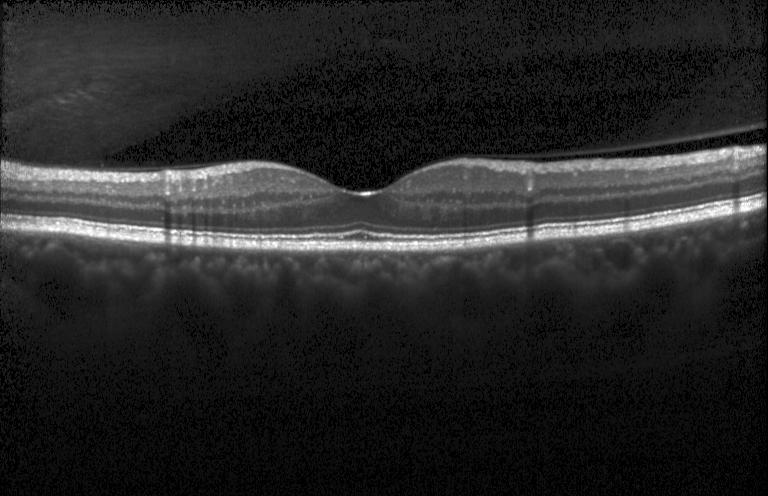 OCT B-scan; spectral-domain optical coherence tomography
Dx: no choroidal neovascularization, diabetic macular edema, or drusen.